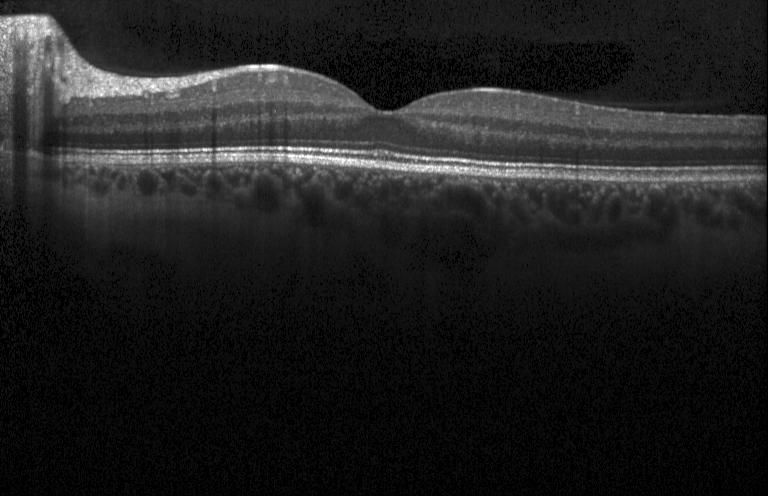 Macular scan. Retinal OCT cross-section — Impression: no evidence of CNV, DME, or drusen.